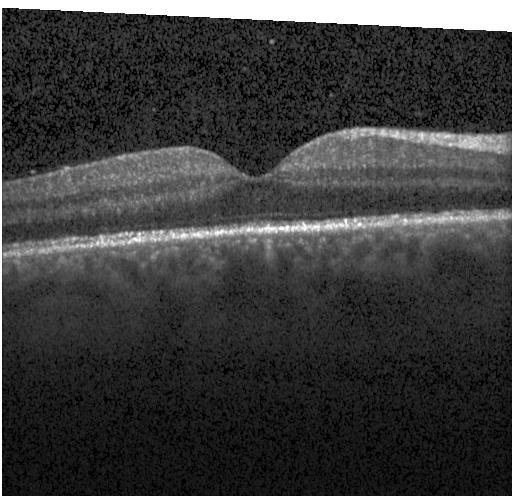
Finding: no evidence of choroidal neovascularization, diabetic macular edema, or drusen.